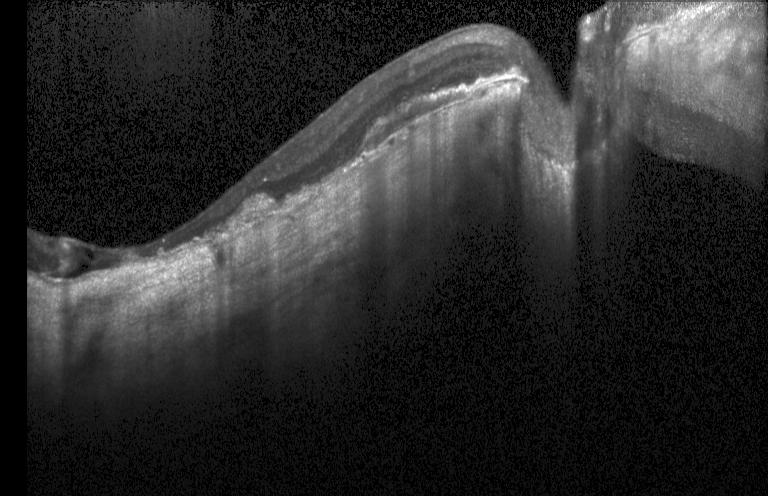

The scan shows a choroidal neovascular membrane.